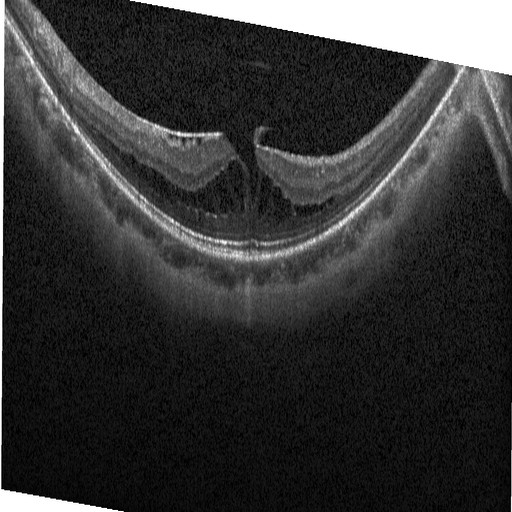 Optical coherence tomography B-scan, macular scan — Finding: DME.